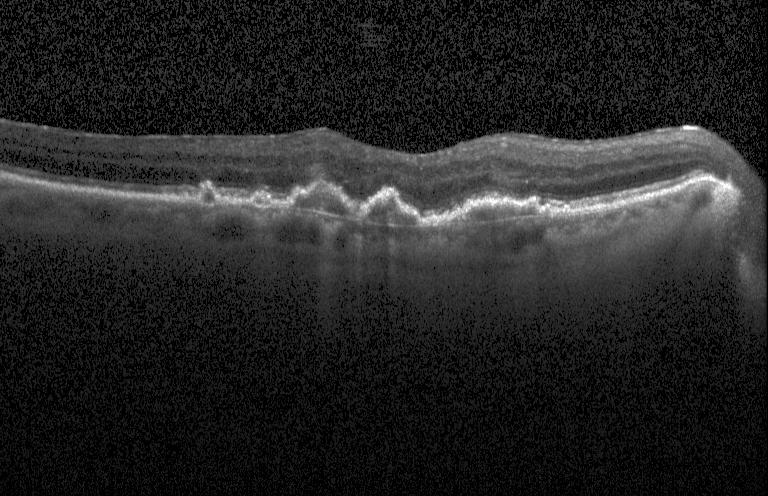 Instrument: Heidelberg Spectralis; spectral-domain optical coherence tomography; optical coherence tomography scan; fovea-centered
A choroidal neovascular membrane.